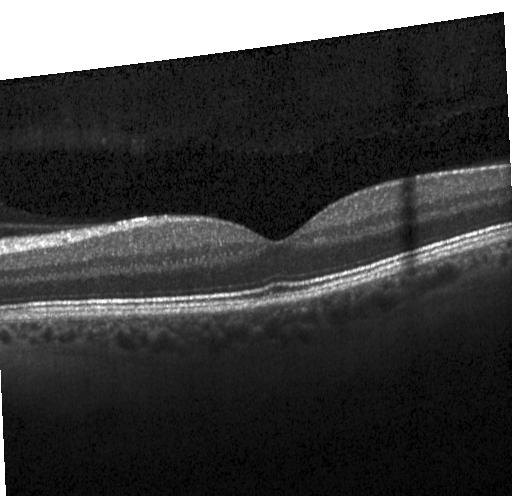 OCT finding: no evidence of choroidal neovascularization, diabetic macular edema, or drusen.